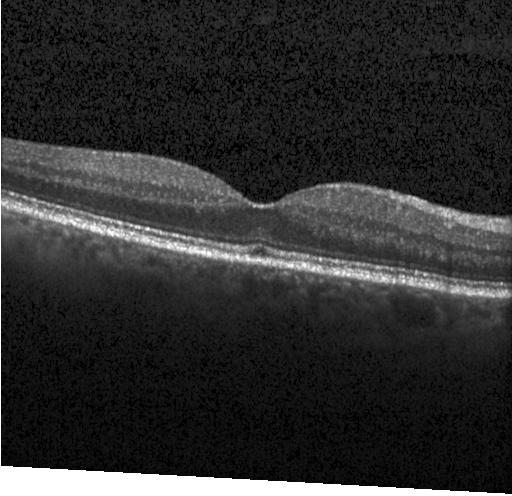

Instrument: Heidelberg Spectralis; centered on the fovea; OCT line scan.
No choroidal neovascularization, no diabetic macular edema, and no drusen.